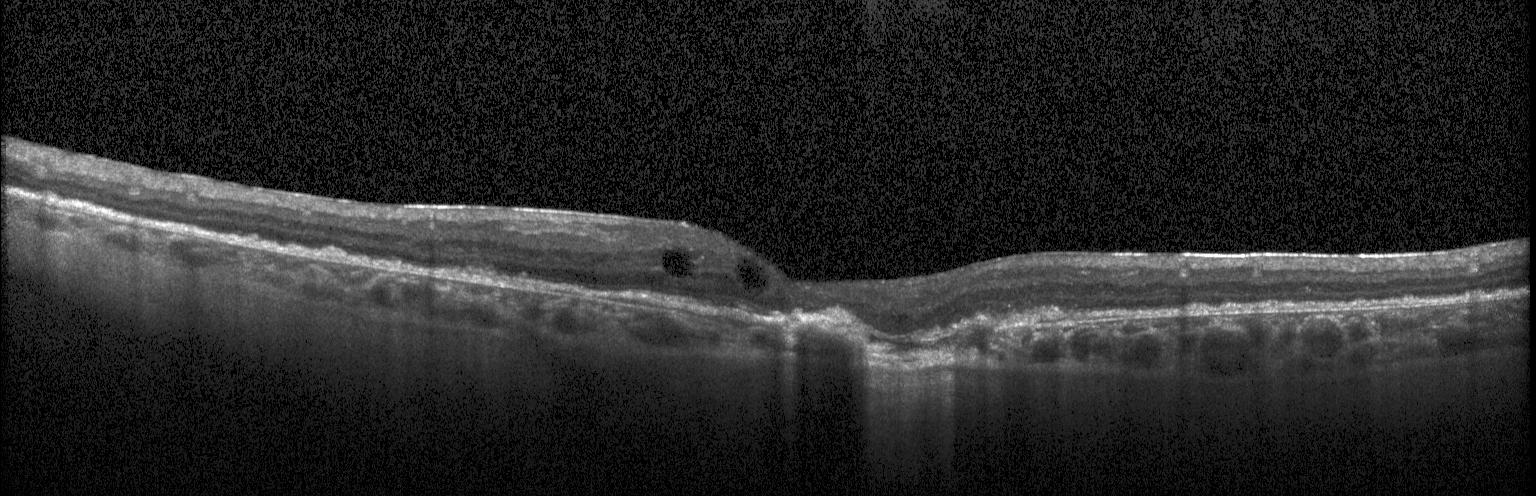 This B-scan demonstrates a choroidal neovascular membrane.